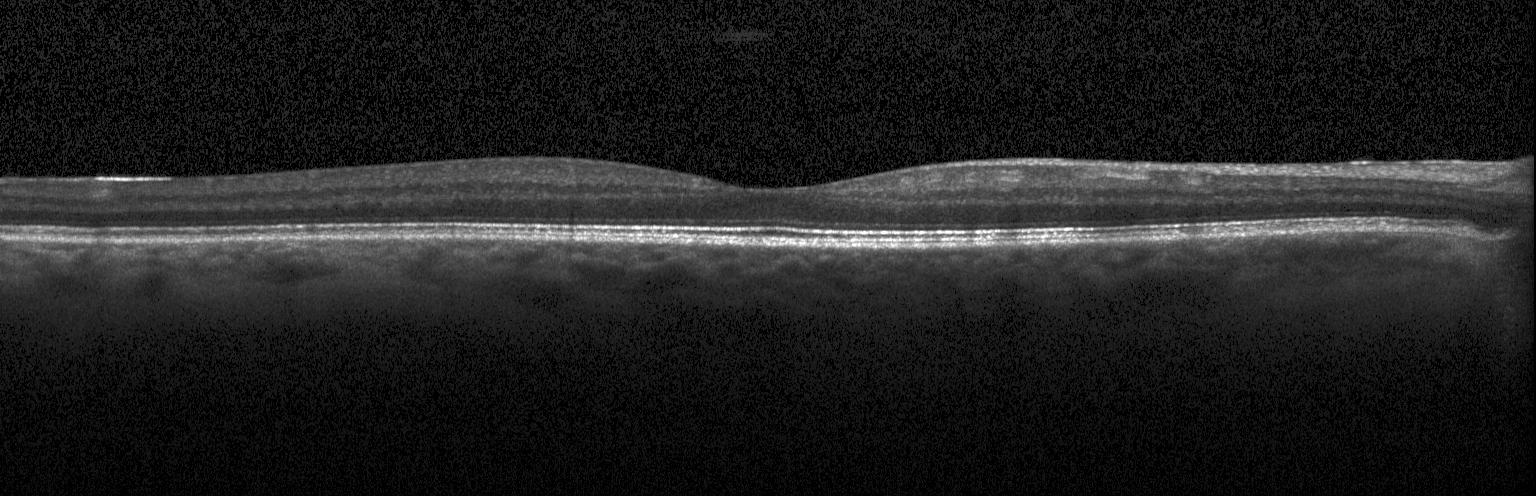

Optical coherence tomography B-scan — Impression: no evidence of choroidal neovascularization, diabetic macular edema, or drusen.